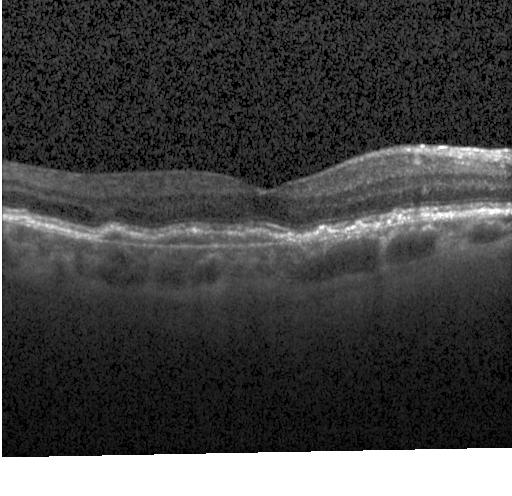
Optical coherence tomography B-scan; macular scan — OCT finding: a choroidal neovascular membrane.